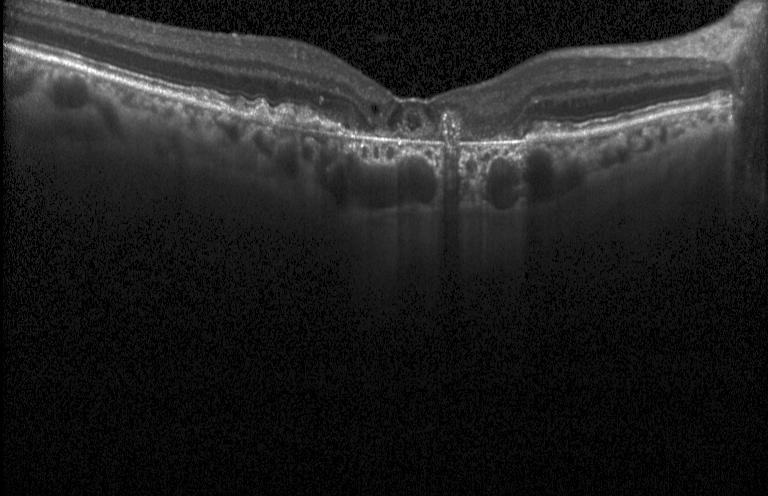

Impression: choroidal neovascularization.